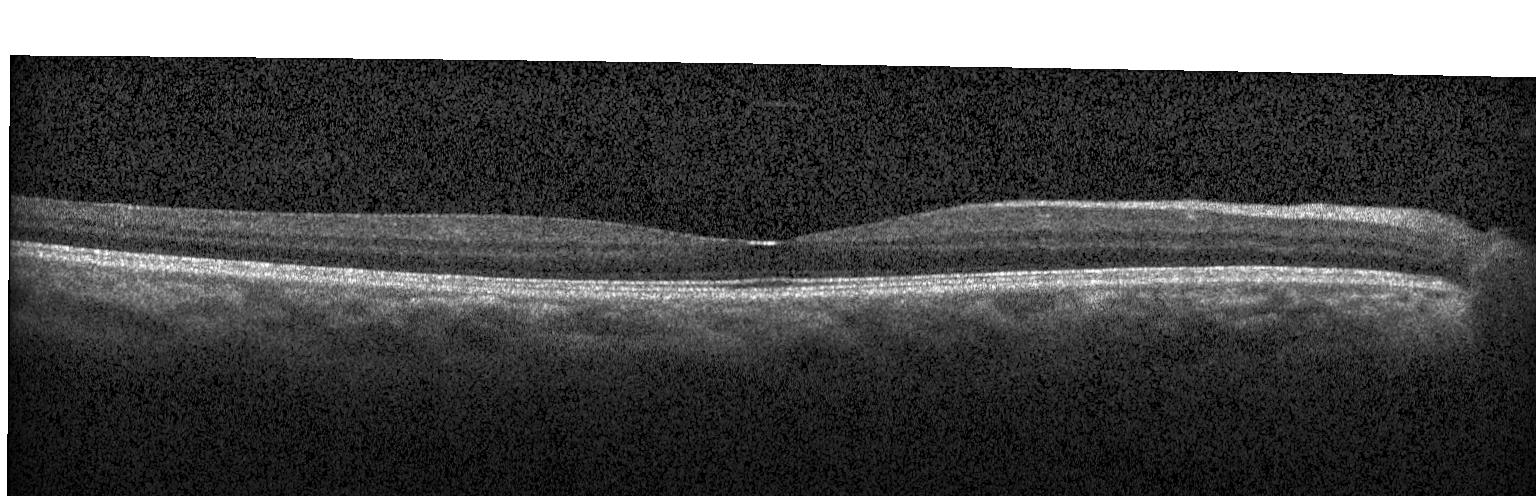 No choroidal neovascularization, no diabetic macular edema, and no drusen.